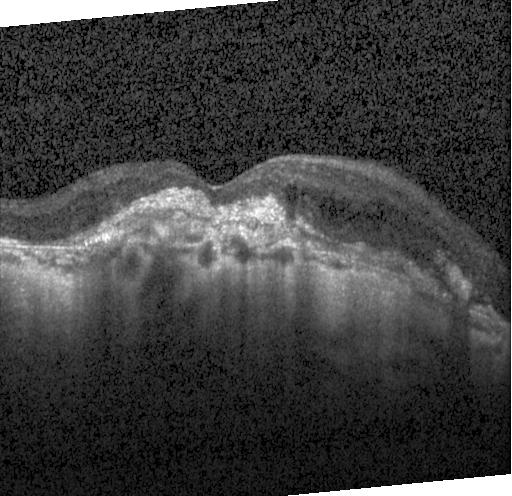
OCT B-scan showing a choroidal neovascular membrane.